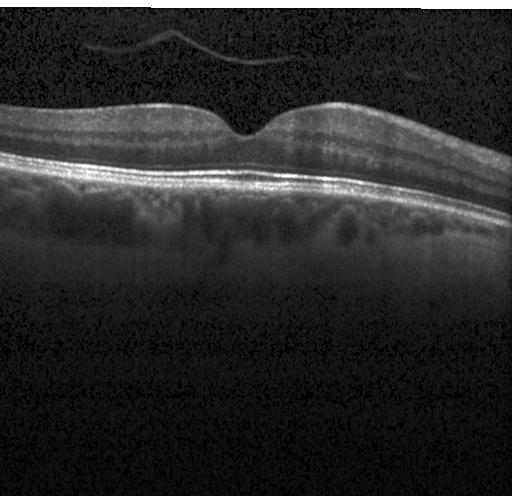 OCT B-scan, spectral-domain optical coherence tomography, horizontal scan through the fovea.
Assessment: no CNV, DME, or drusen.